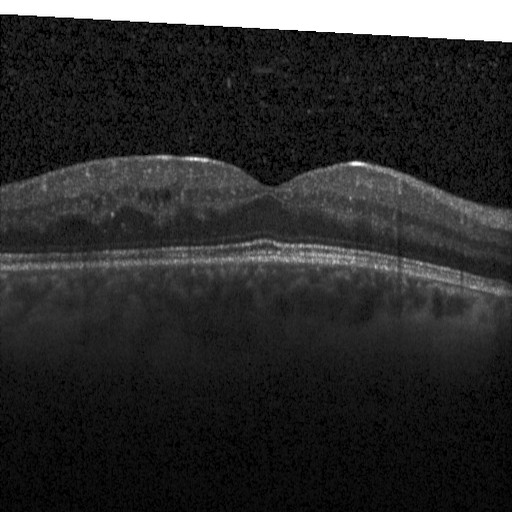 Dx: diabetic macular edema.